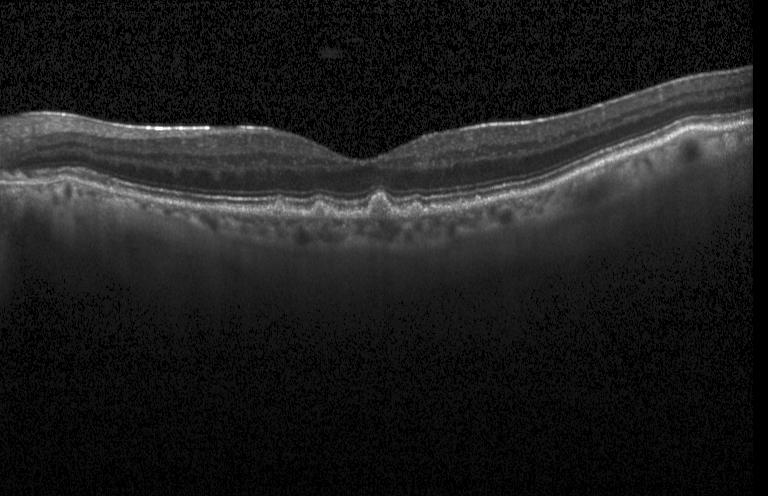 OCT B-scan. Impression: sub-RPE drusenoid deposits.